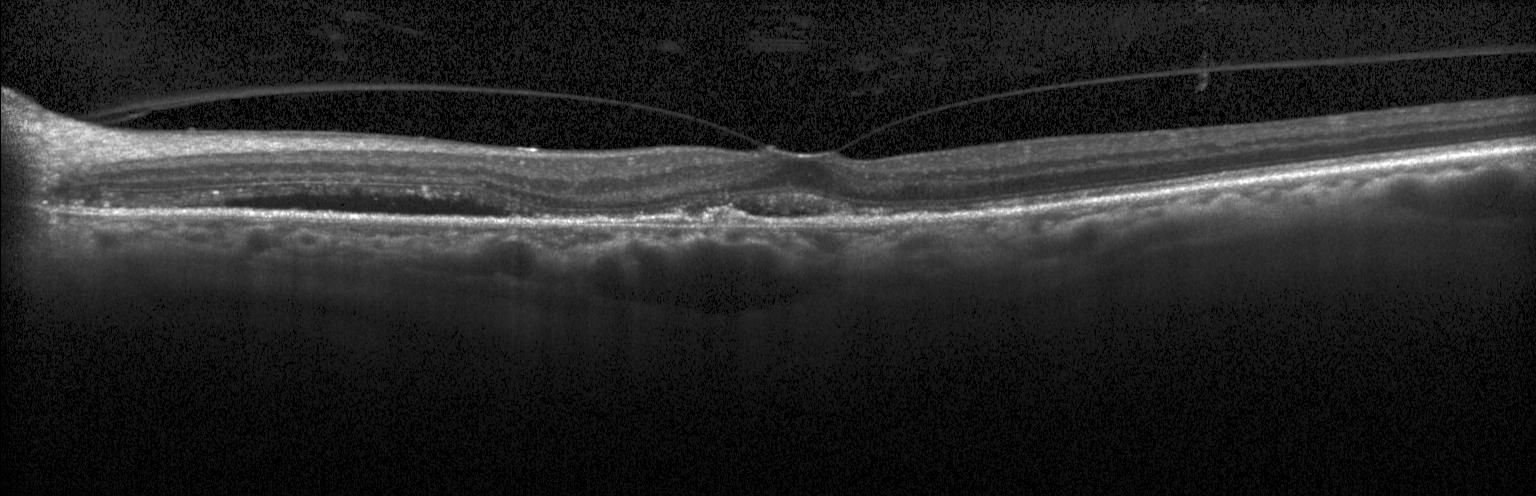
Dx: choroidal neovascularization (CNV).